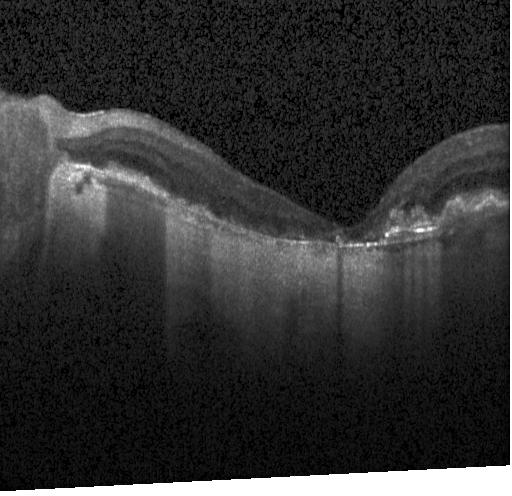

Spectral-domain OCT. Heidelberg Spectralis OCT system. Retinal OCT cross-section — The scan shows CNV.